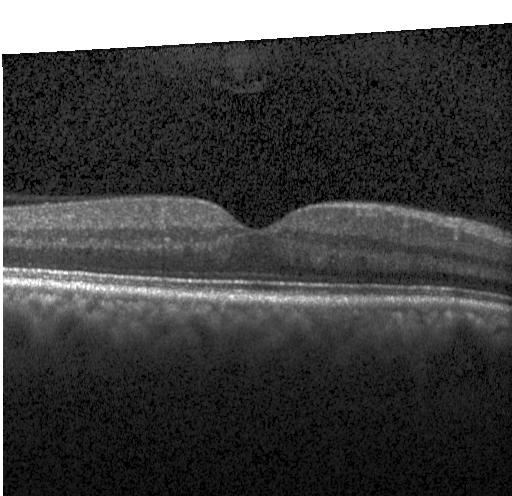

The scan shows no CNV, no DME, and no drusen.